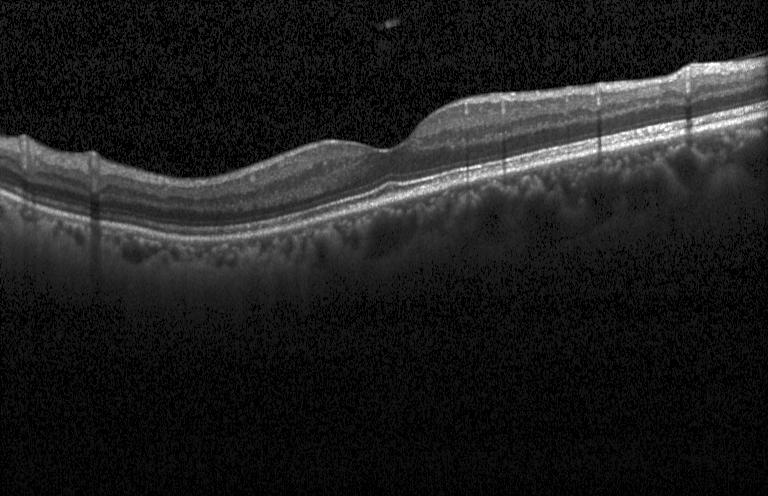

OCT line scan — The scan shows no evidence of CNV, DME, or drusen.